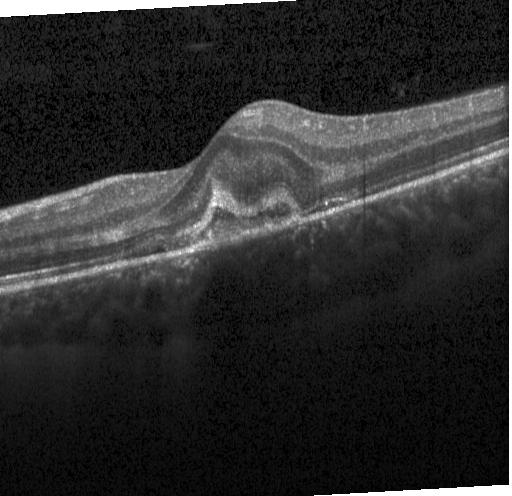 Centered on the fovea; spectral-domain OCT; acquired on a Heidelberg Spectralis; OCT B-scan — Impression: a choroidal neovascular membrane.